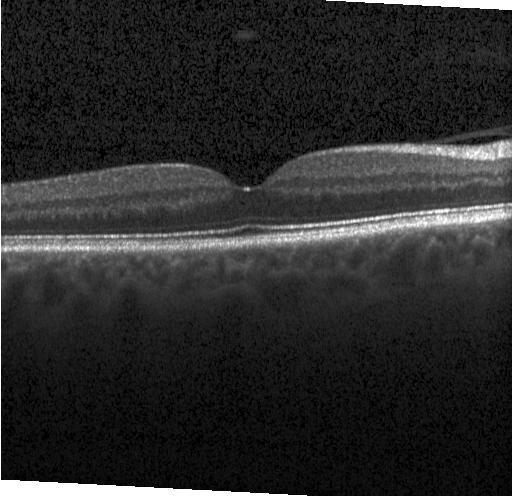

Horizontal scan through the fovea. Optical coherence tomography B-scan.
Finding: no CNV, DME, or drusen.